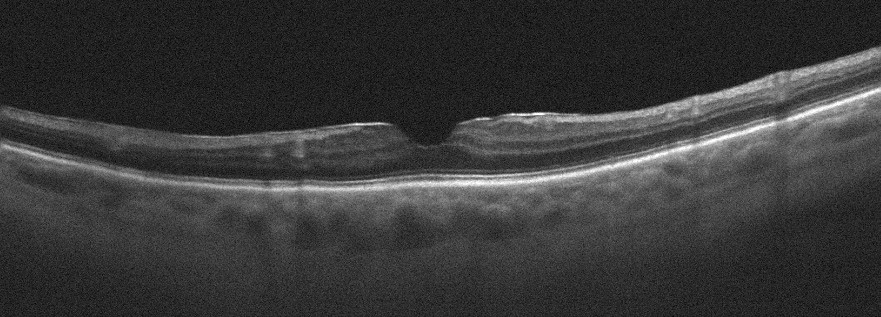 OCT B-scan — Finding: epiretinal membrane.